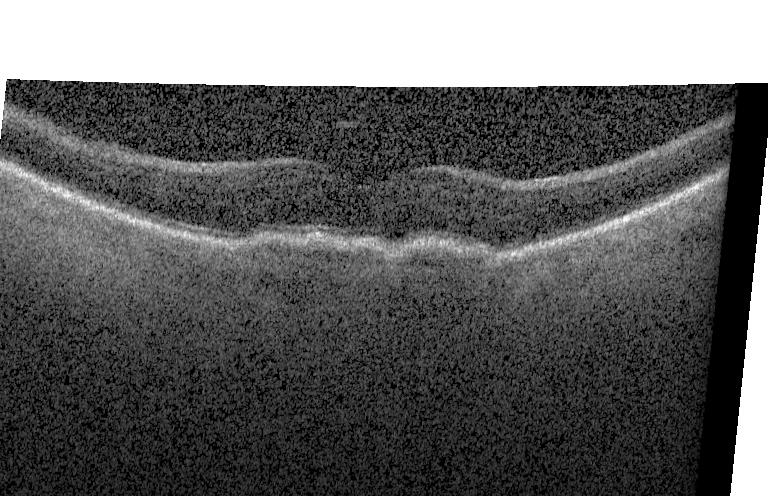 Retinal OCT cross-section showing a choroidal neovascular membrane.